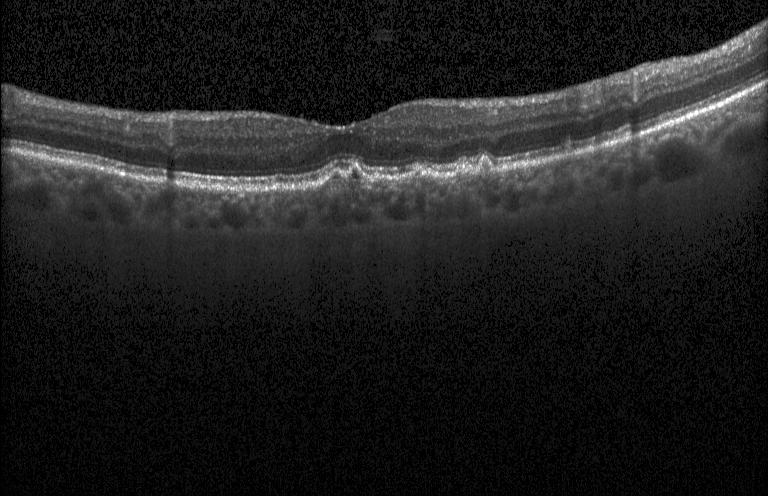

Dx: multiple drusen.